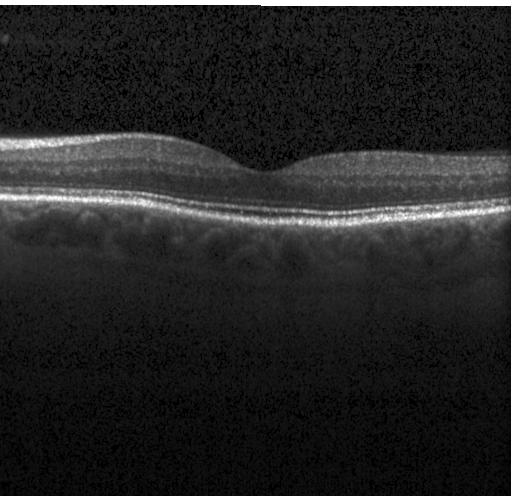

Spectral-domain OCT. OCT B-scan
Assessment: no CNV, no DME, and no drusen.